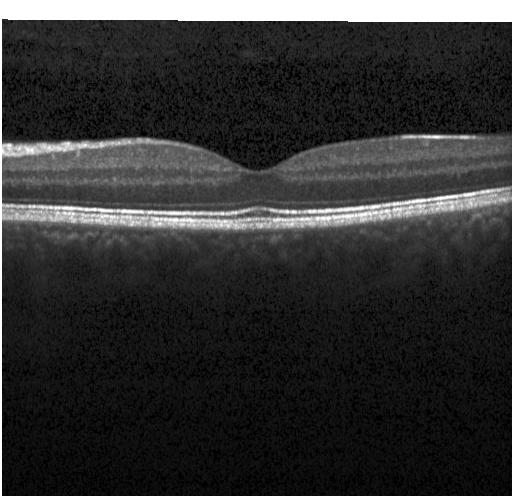
Diagnosis: no choroidal neovascularization, no diabetic macular edema, and no drusen.